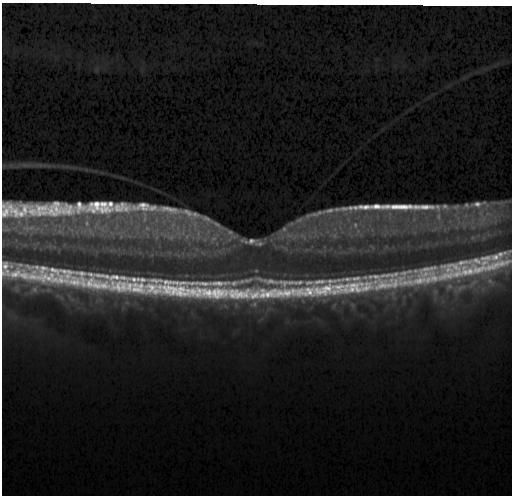 Optical coherence tomography B-scan
This B-scan demonstrates no choroidal neovascularization, no diabetic macular edema, and no drusen.